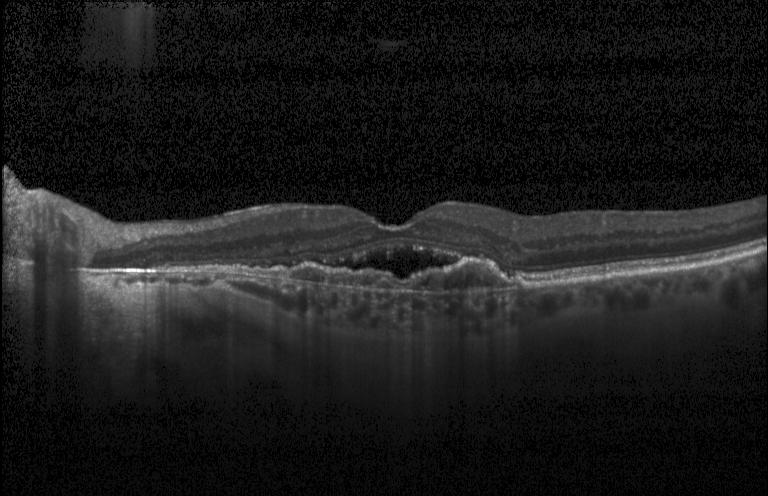 Finding: CNV.